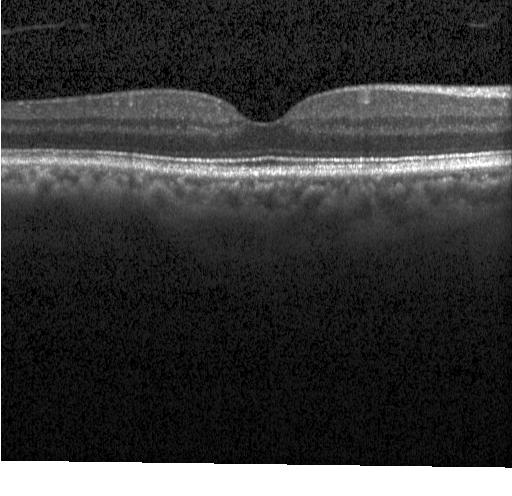

Assessment: neither choroidal neovascularization, diabetic macular edema, nor drusen.